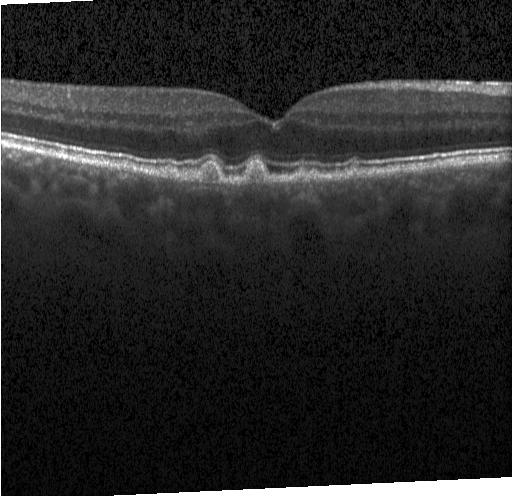 Dx: sub-RPE drusenoid deposits.